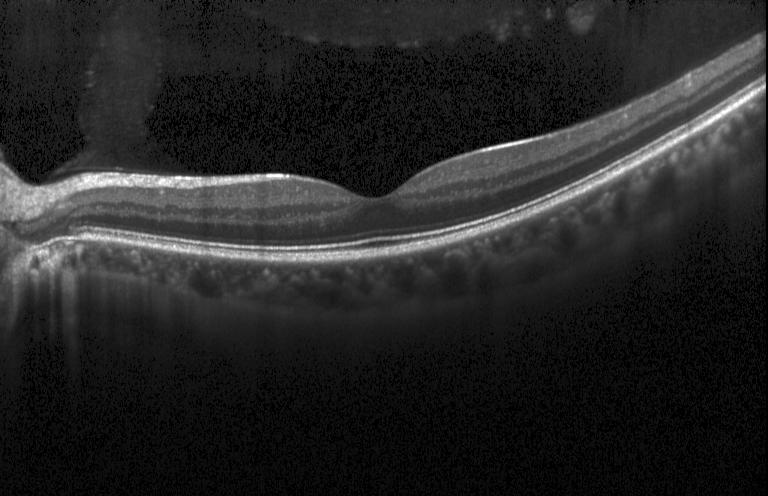
The scan shows no choroidal neovascularization, diabetic macular edema, or drusen.